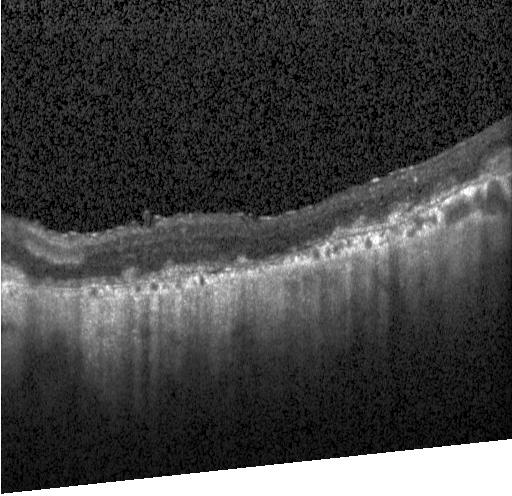
Impression: choroidal neovascularization (CNV).